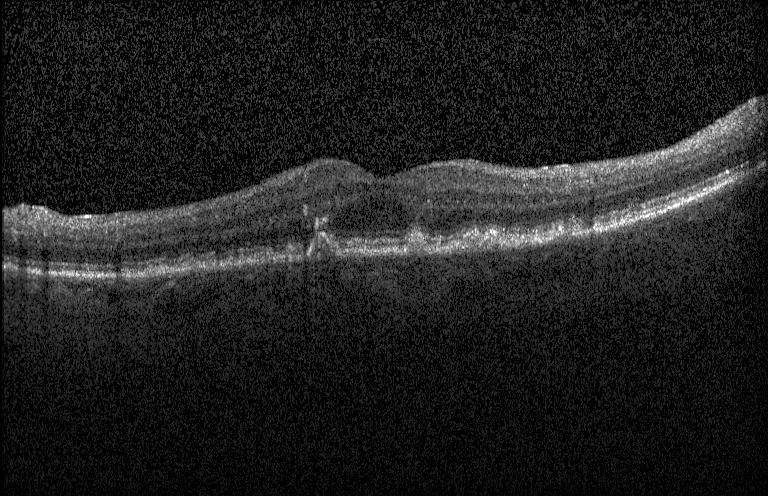
OCT finding: multiple drusen.